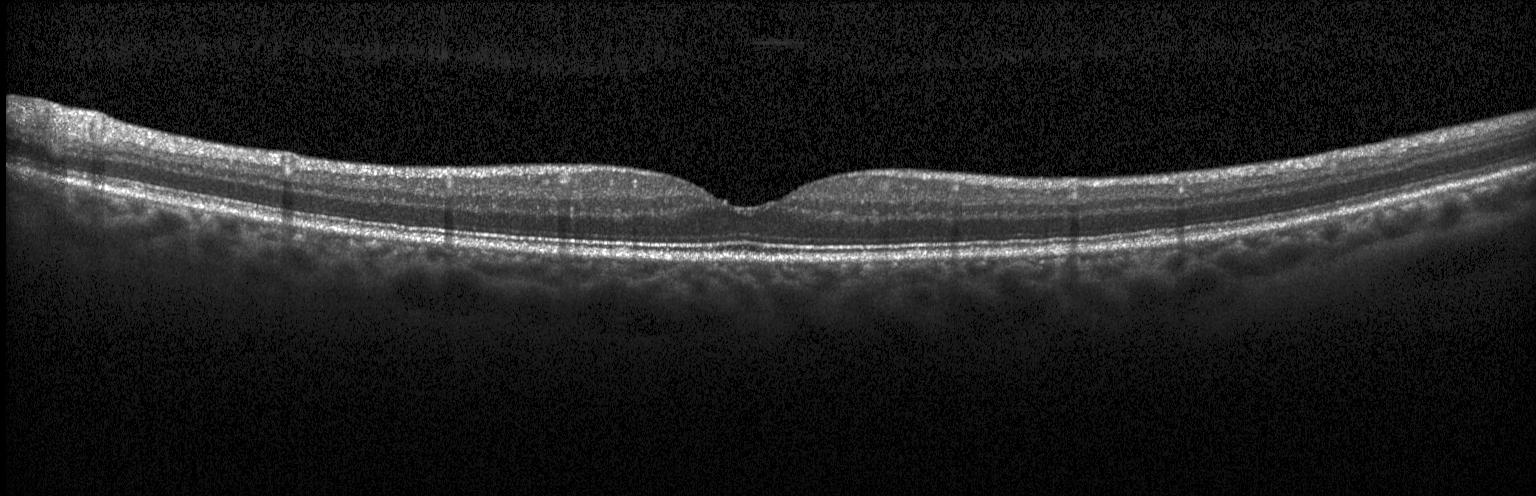 OCT B-scan, Heidelberg Spectralis OCT system, SD-OCT, centered on the fovea.
Impression: no choroidal neovascularization, diabetic macular edema, or drusen.